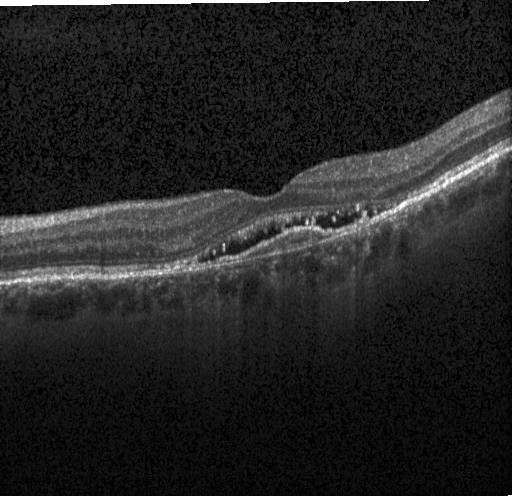

OCT B-scan showing choroidal neovascularization.